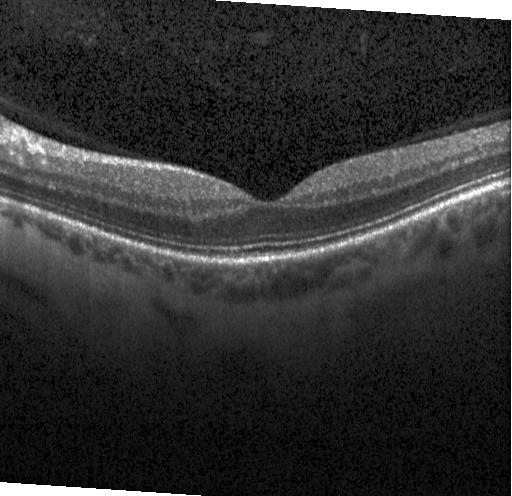

OCT B-scan; spectral-domain optical coherence tomography; acquired on a Heidelberg Spectralis. Diagnosis: no choroidal neovascularization, diabetic macular edema, or drusen.